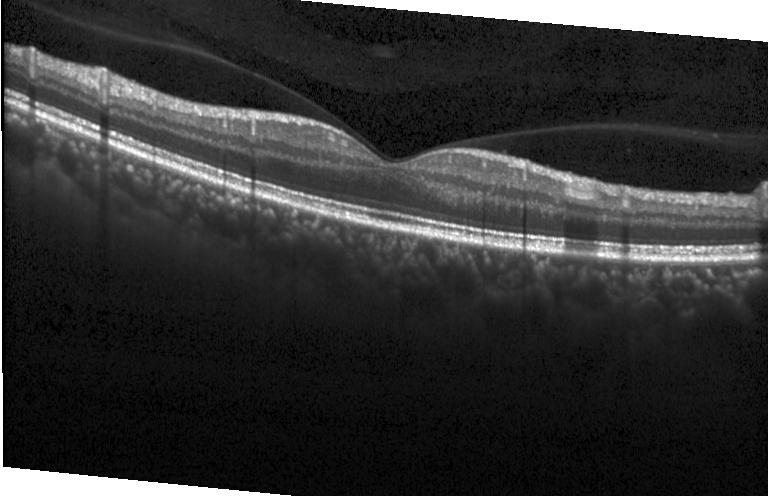
This B-scan demonstrates neither CNV, DME, nor drusen.